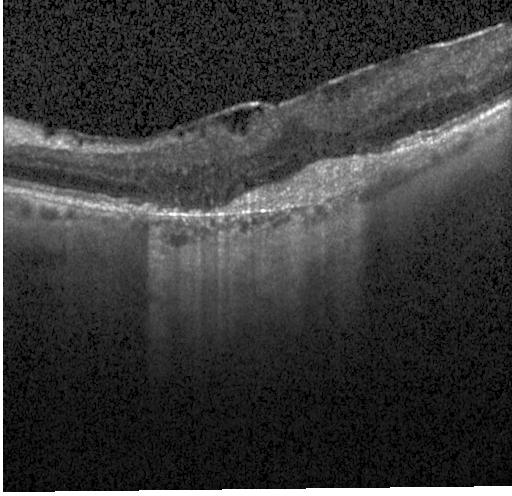

SD-OCT; optical coherence tomography B-scan.
Diagnosis: a choroidal neovascular membrane.